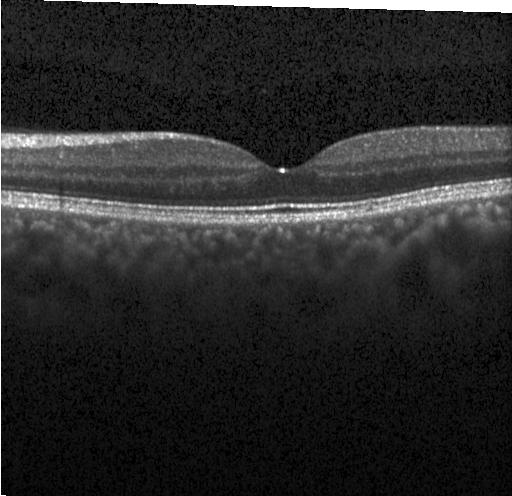 Optical coherence tomography B-scan, macular scan, spectral-domain OCT, Heidelberg Spectralis OCT system
Dx: no choroidal neovascularization, diabetic macular edema, or drusen.